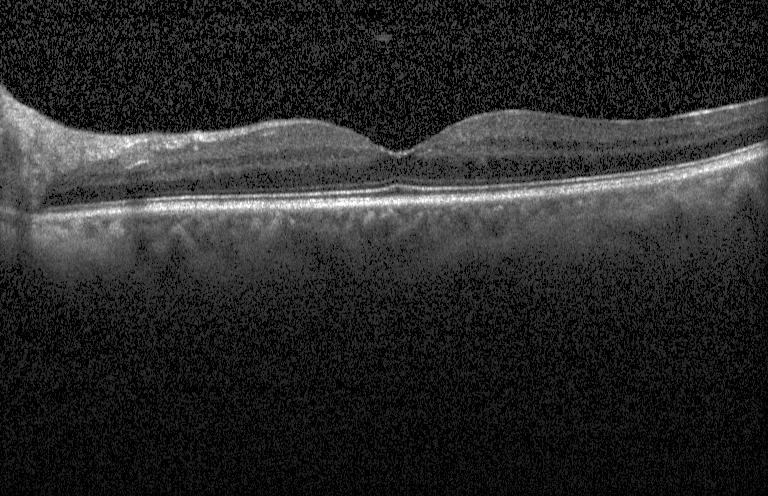

Optical coherence tomography scan. Diagnosis: no CNV, no DME, and no drusen.